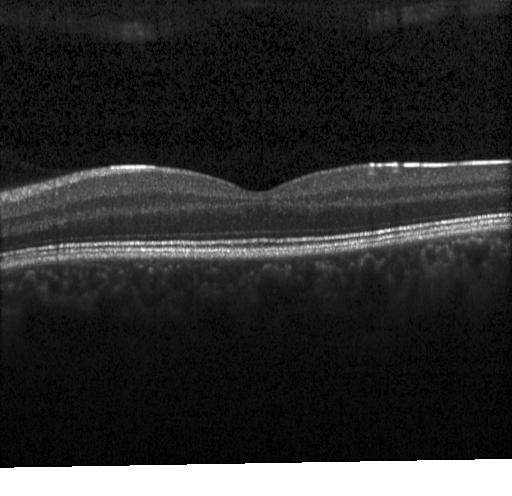

Retinal OCT B-scan, spectral-domain OCT — The scan shows no choroidal neovascularization, diabetic macular edema, or drusen.